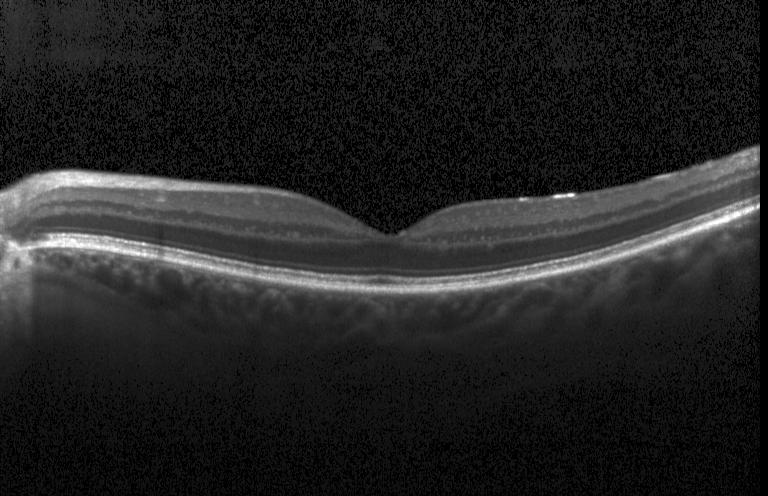

Optical coherence tomography B-scan. Fovea-centered. Heidelberg Spectralis OCT system.
OCT finding: no CNV, DME, or drusen.